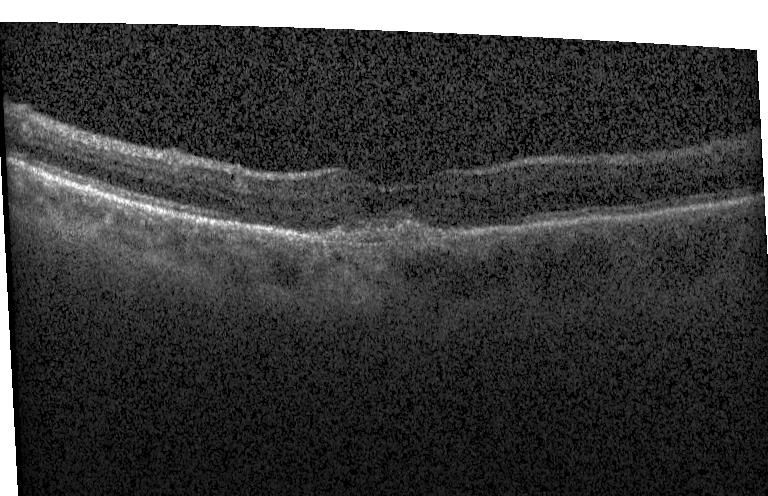
Diagnosis: a choroidal neovascular membrane.